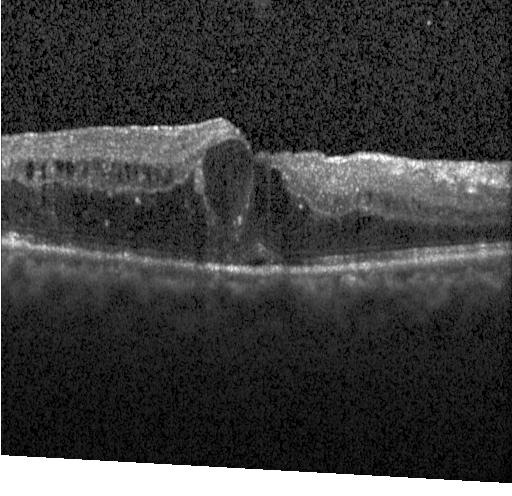
Impression: diabetic macular edema (DME).